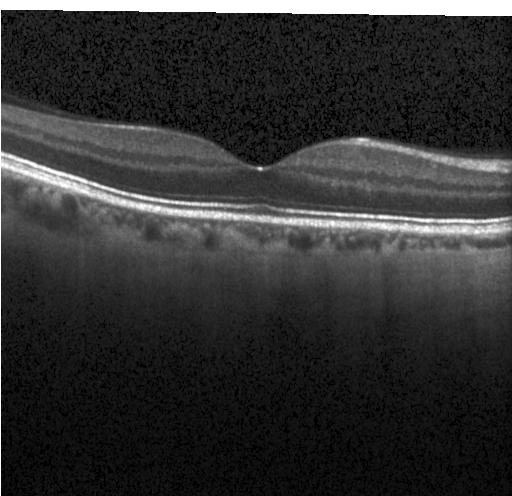 Optical coherence tomography scan.
No CNV, no DME, and no drusen.